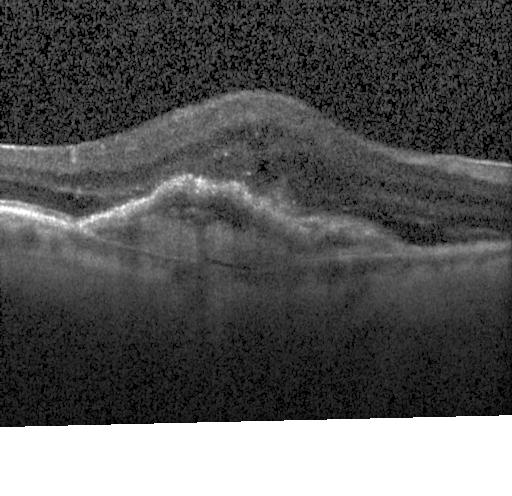

Heidelberg Spectralis OCT system · retinal OCT cross-section — Impression: choroidal neovascularization.